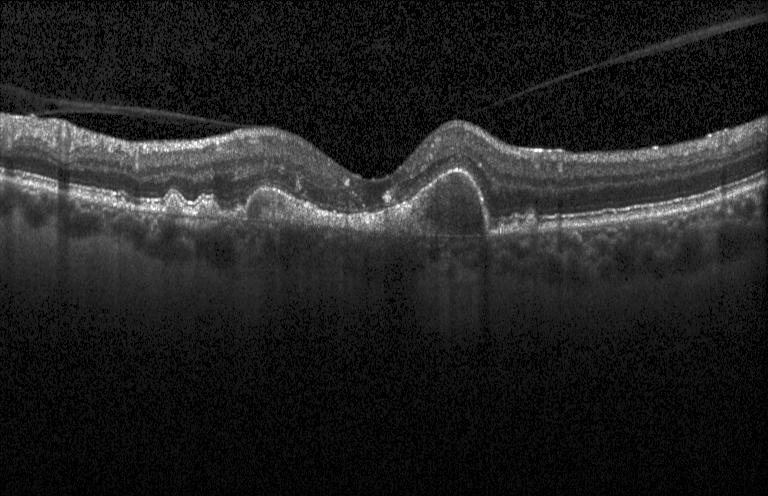
OCT finding: CNV.